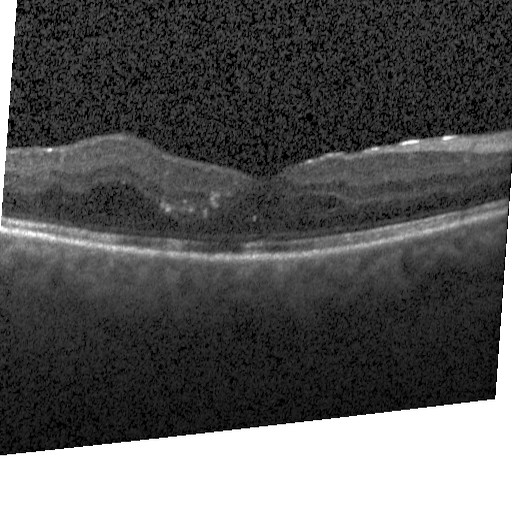
Spectral-domain optical coherence tomography; OCT B-scan; macular scan — Dx: DME.